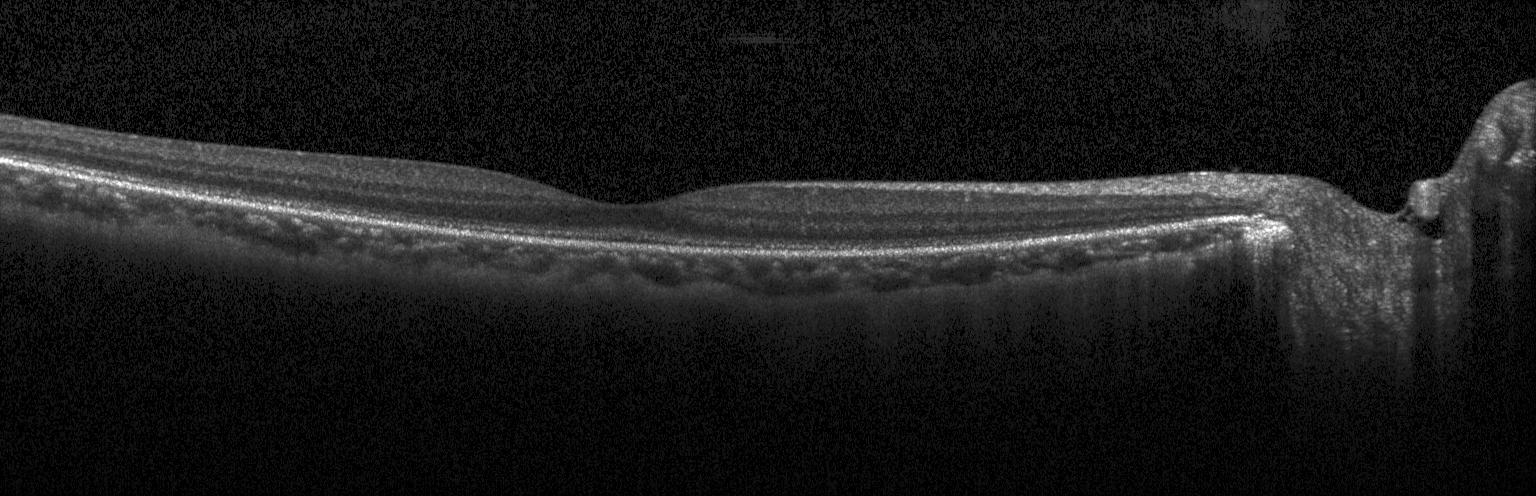 Optical coherence tomography scan
Finding: no choroidal neovascularization, no diabetic macular edema, and no drusen.